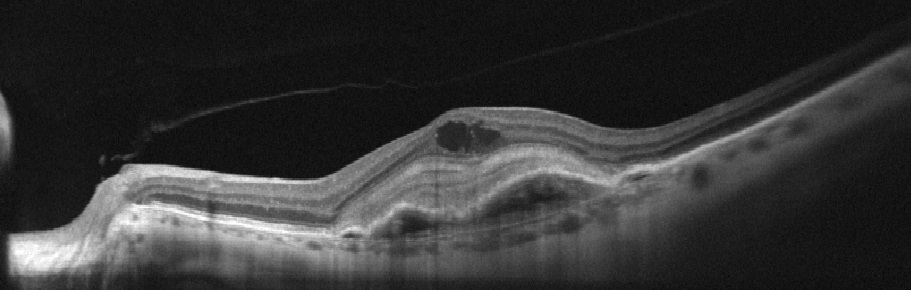

Spectral-domain OCT B-scan: AMD.